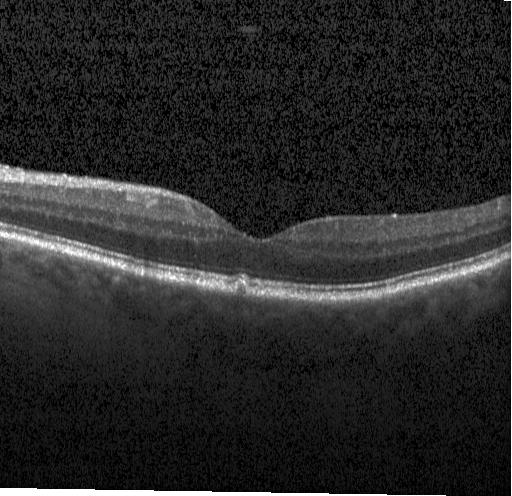

Dx: drusen.